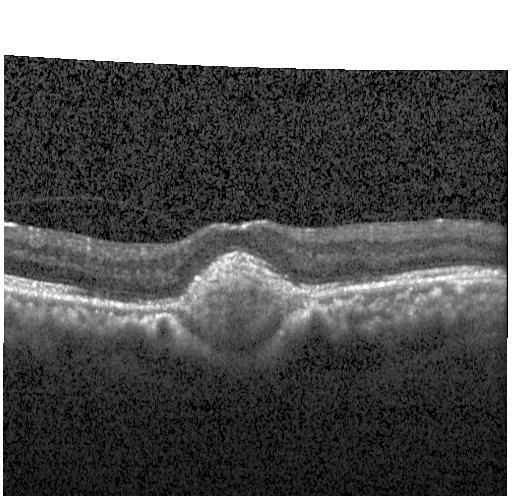

Finding: a choroidal neovascular membrane.